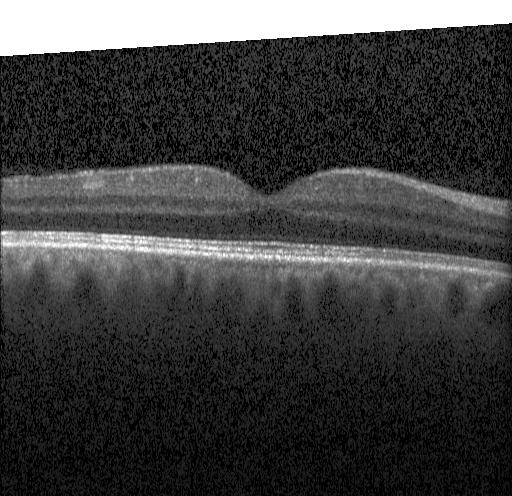
Horizontal scan through the fovea; spectral-domain optical coherence tomography; OCT line scan. Diagnosis: neither choroidal neovascularization, diabetic macular edema, nor drusen.